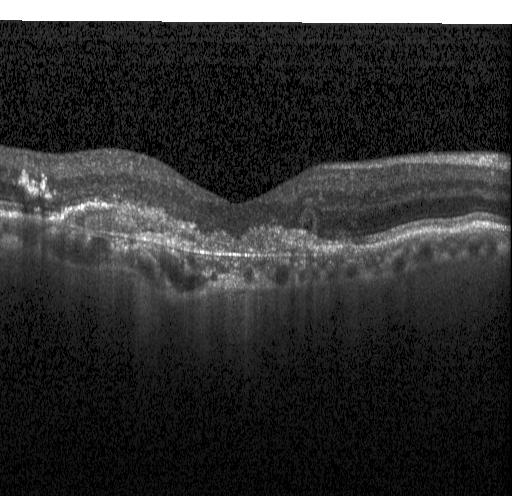

Assessment: CNV.